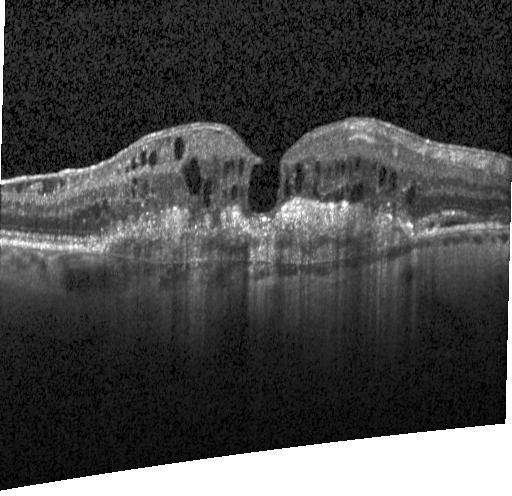
Spectral-domain optical coherence tomography, retinal OCT cross-section
Diagnosis: CNV.